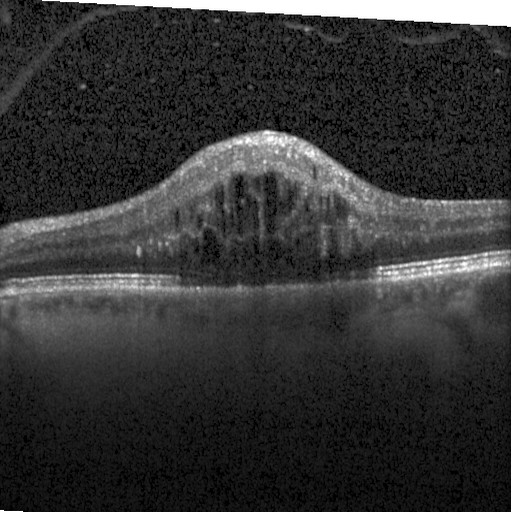

Diabetic macular edema.